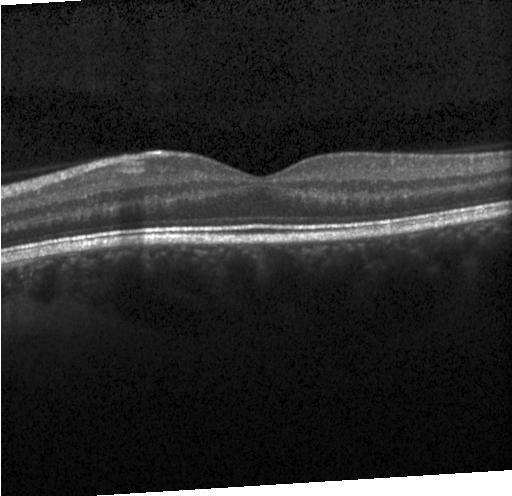

Impression: neither choroidal neovascularization, diabetic macular edema, nor drusen.